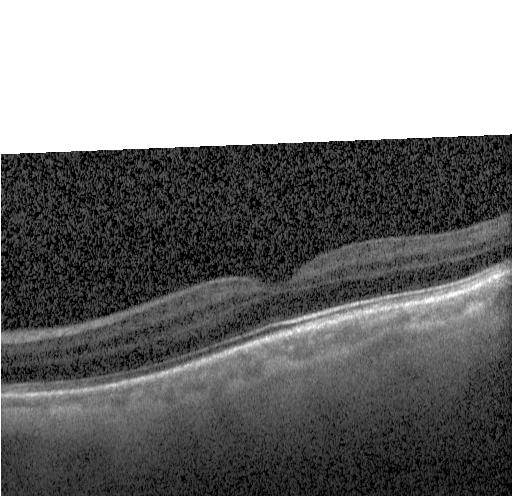

OCT B-scan. Spectral-domain OCT
The scan shows neither choroidal neovascularization, diabetic macular edema, nor drusen.